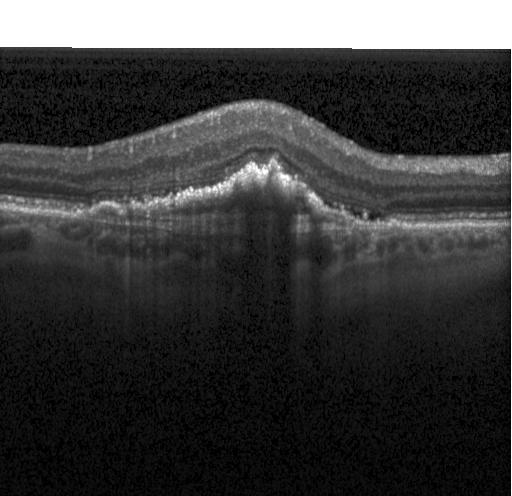
Heidelberg Spectralis OCT system; SD-OCT; macular scan; OCT line scan
Dx: choroidal neovascularization (CNV).